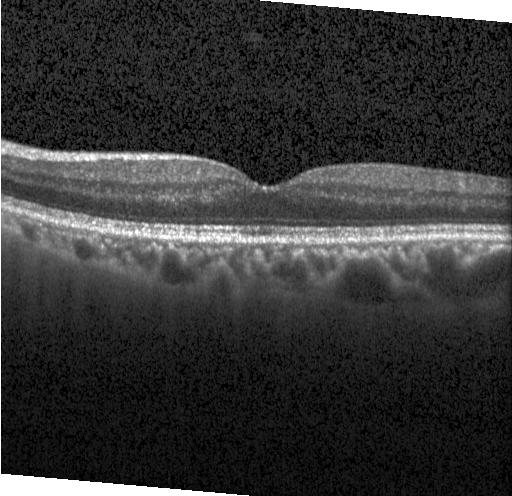

Instrument: Heidelberg Spectralis. SD-OCT. Retinal OCT B-scan
Diagnosis: no choroidal neovascularization, no diabetic macular edema, and no drusen.